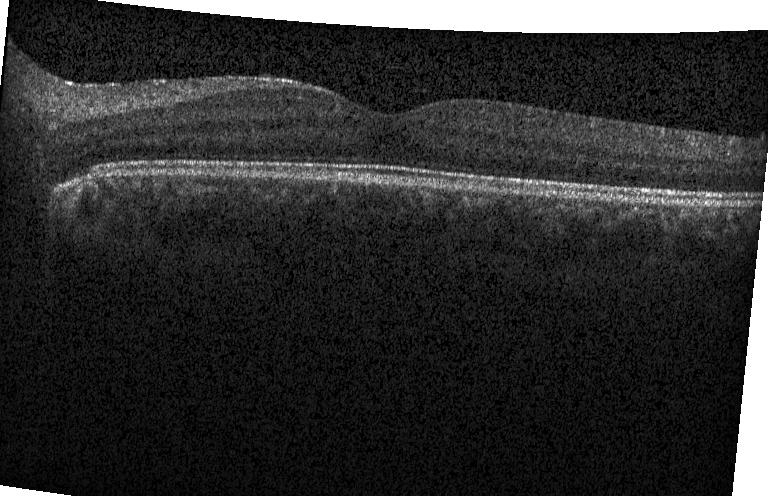

Instrument: Heidelberg Spectralis, retinal OCT cross-section, SD-OCT. Neither choroidal neovascularization, diabetic macular edema, nor drusen.